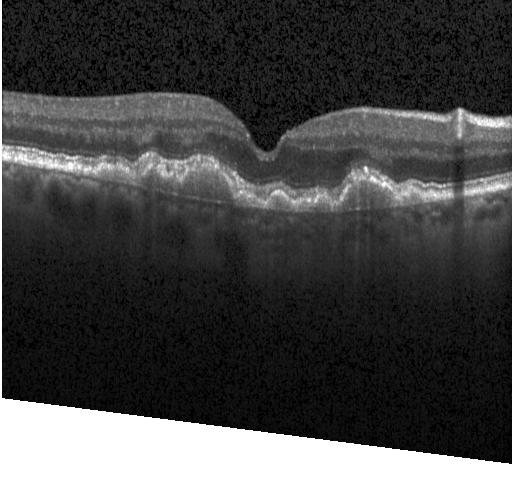 Finding: sub-RPE drusenoid deposits.